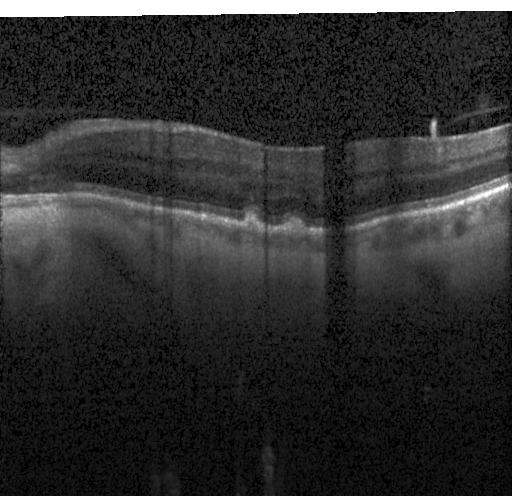
Horizontal scan through the fovea · acquired on a Heidelberg Spectralis · spectral-domain optical coherence tomography · OCT B-scan
Assessment: multiple drusen.